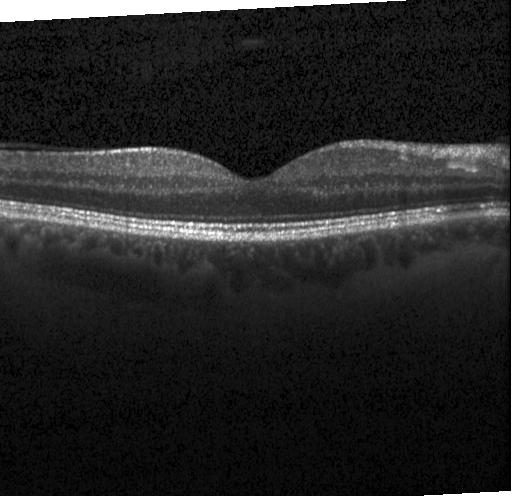

Diagnosis: no choroidal neovascularization, diabetic macular edema, or drusen.